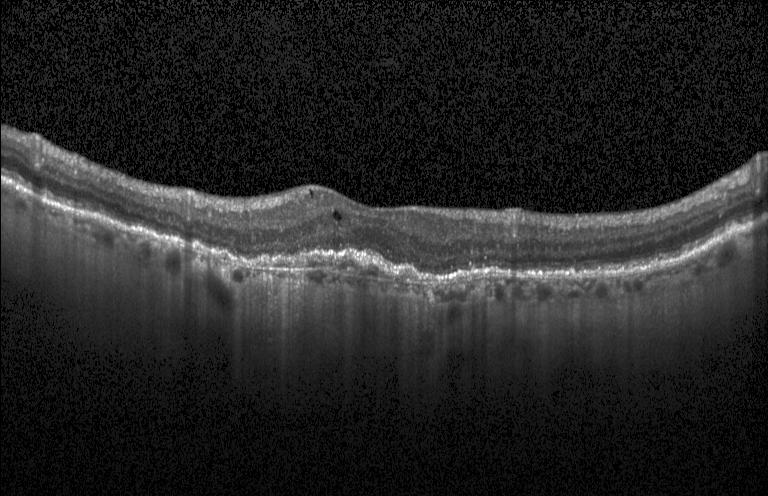 Heidelberg Spectralis. OCT line scan. SD-OCT. Centered on the fovea
Diagnosis: choroidal neovascularization (CNV).